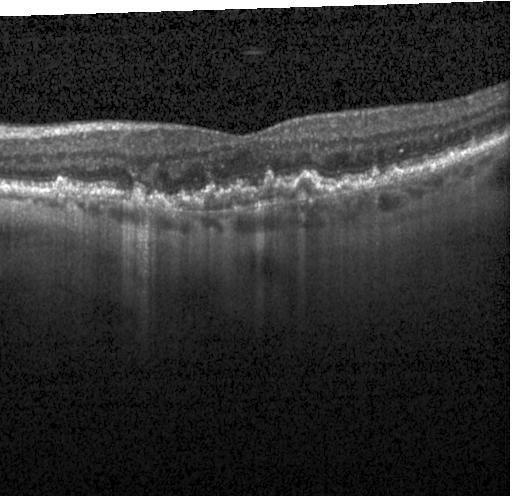
Heidelberg Spectralis, spectral-domain optical coherence tomography, OCT B-scan. Assessment: CNV.